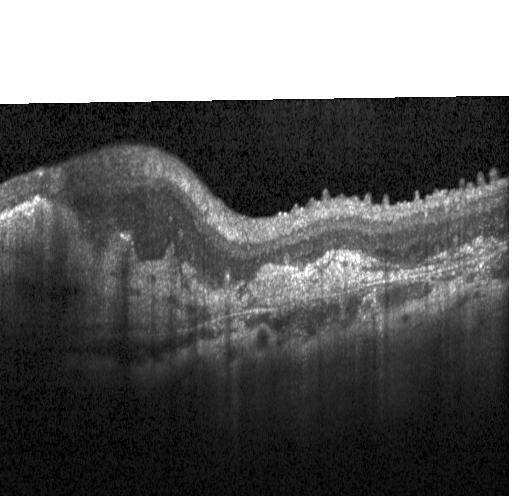
Centered on the fovea, SD-OCT, Heidelberg Spectralis, retinal OCT cross-section
Impression: choroidal neovascularization (CNV).